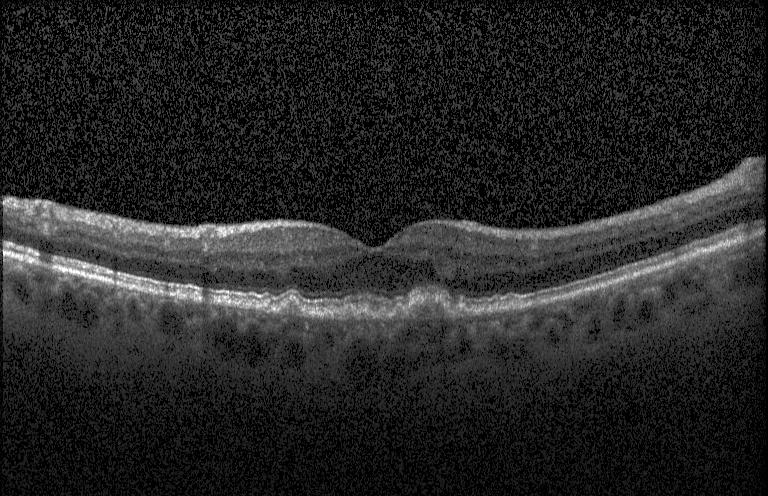
Heidelberg Spectralis · centered on the fovea · OCT line scan.
Dx: drusen.